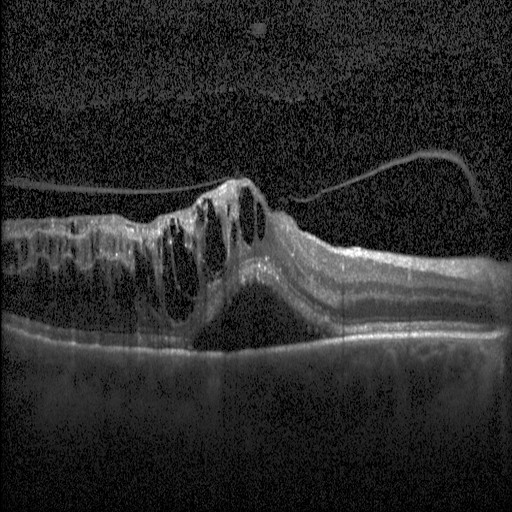 Retinal OCT cross-section. The scan shows DME.